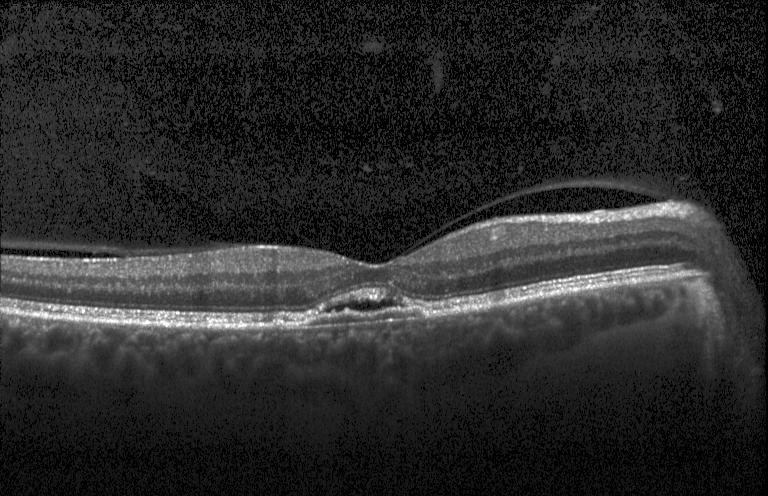
OCT line scan
Macular OCT: CNV.